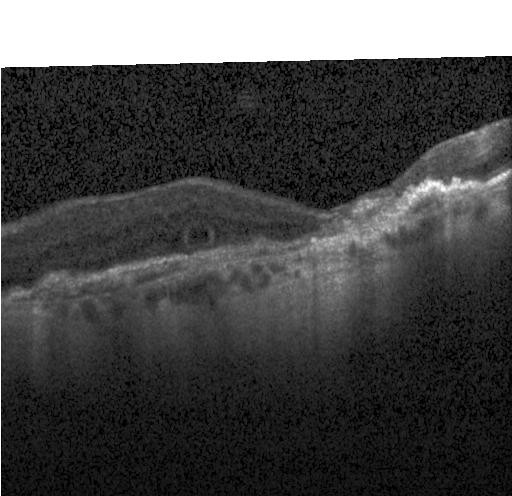
Retinal OCT cross-section; SD-OCT — Diagnosis: CNV.